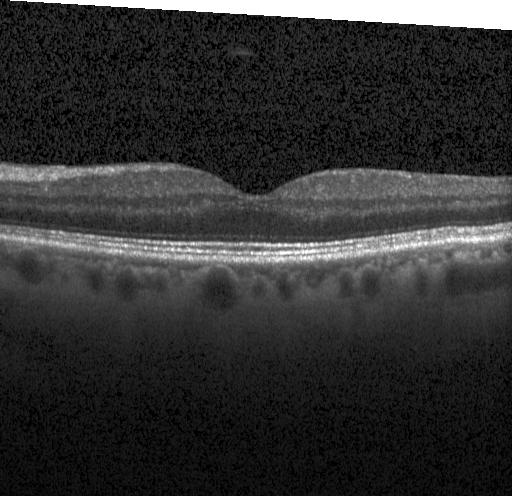

Optical coherence tomography scan. The scan shows no CNV, no DME, and no drusen.